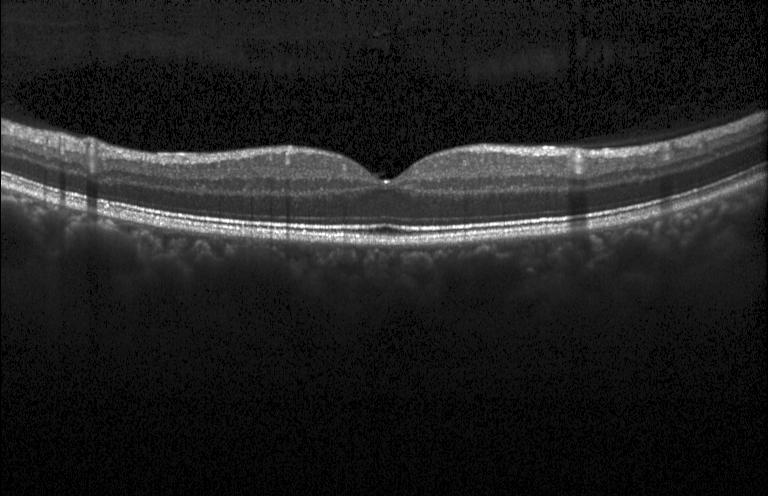
Optical coherence tomography scan; SD-OCT; acquired on a Heidelberg Spectralis; macular scan
Diagnosis: no CNV, DME, or drusen.